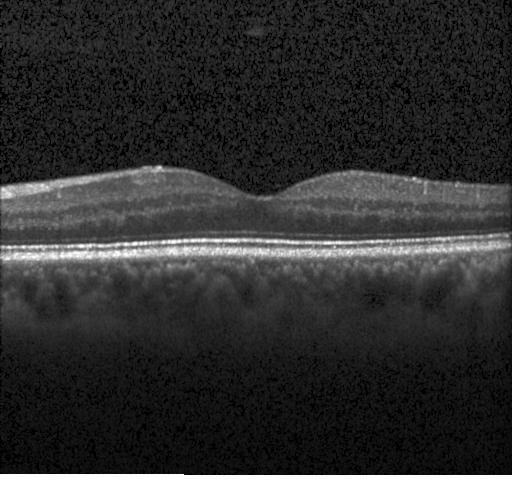
Optical coherence tomography B-scan
Diagnosis: no CNV, no DME, and no drusen.